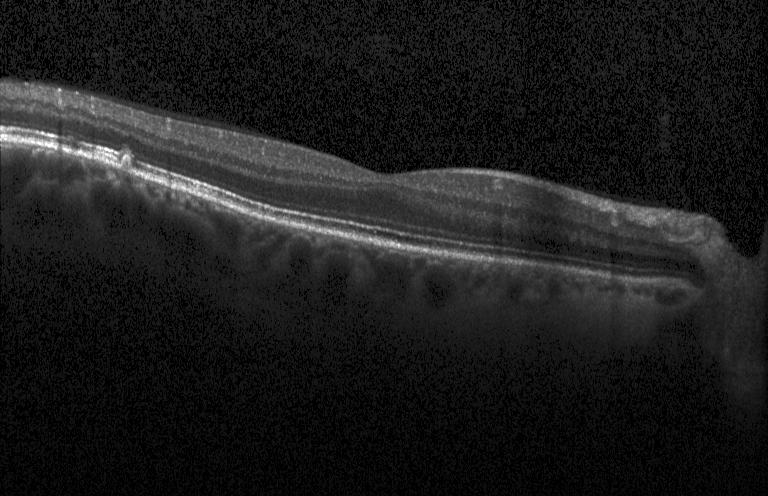
OCT B-scan
Dx: multiple drusen.